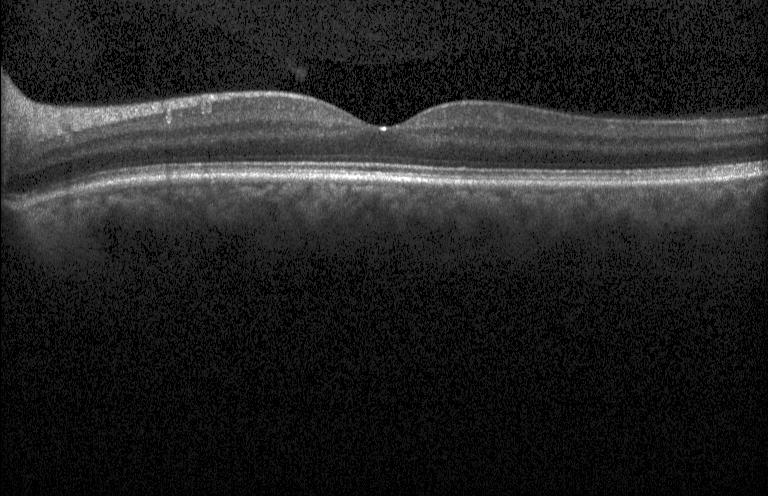
Optical coherence tomography scan; acquired on a Heidelberg Spectralis; spectral-domain optical coherence tomography; macular scan — OCT finding: no choroidal neovascularization, diabetic macular edema, or drusen.